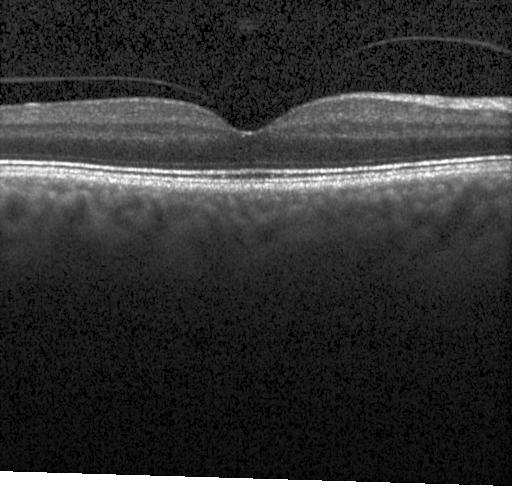 This B-scan demonstrates no CNV, no DME, and no drusen.